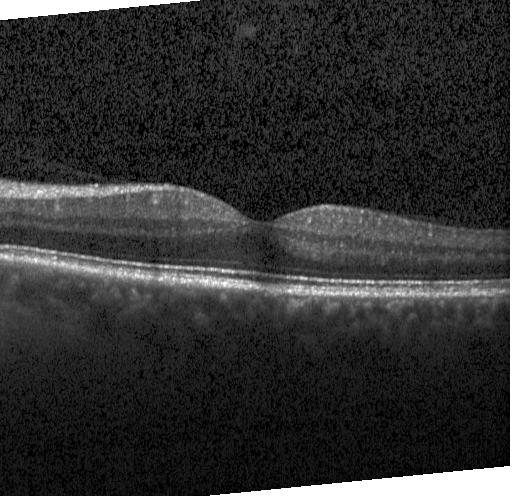

Assessment: neither choroidal neovascularization, diabetic macular edema, nor drusen.